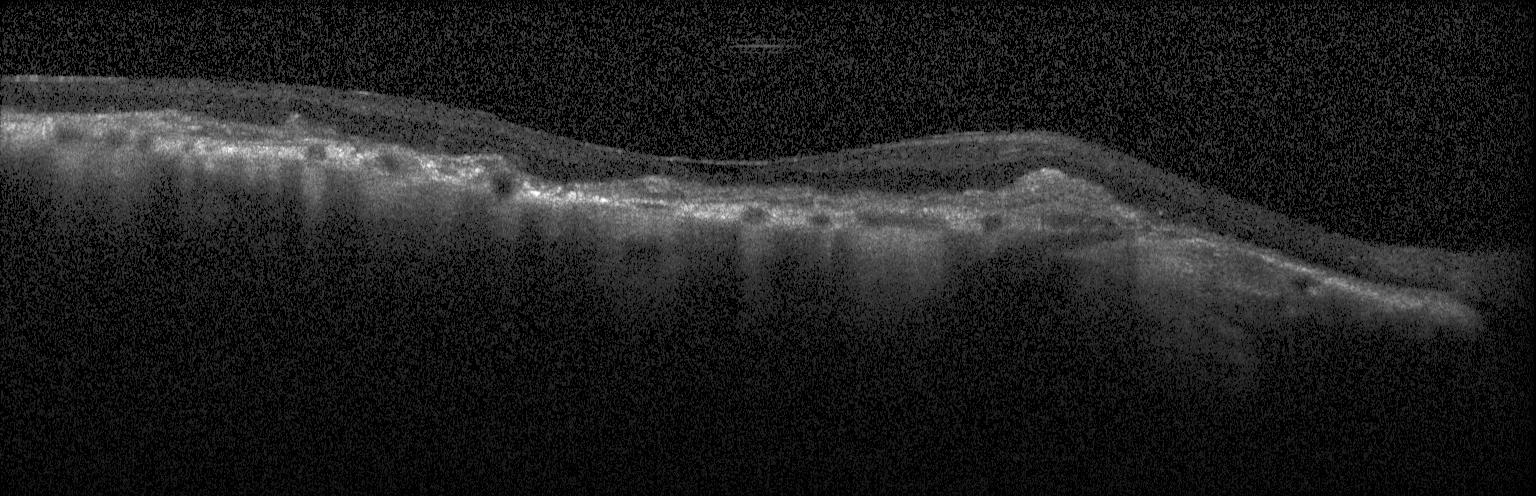 OCT scan showing a choroidal neovascular membrane.